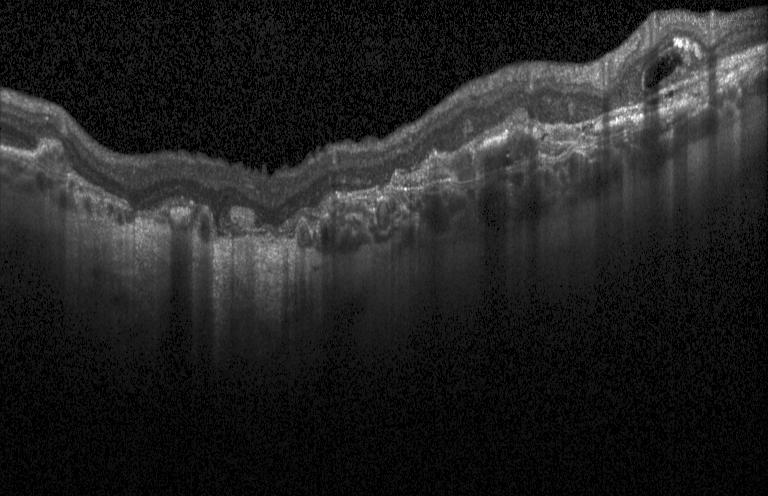
Retinal OCT cross-section; horizontal scan through the fovea; spectral-domain optical coherence tomography. Impression: choroidal neovascularization (CNV).